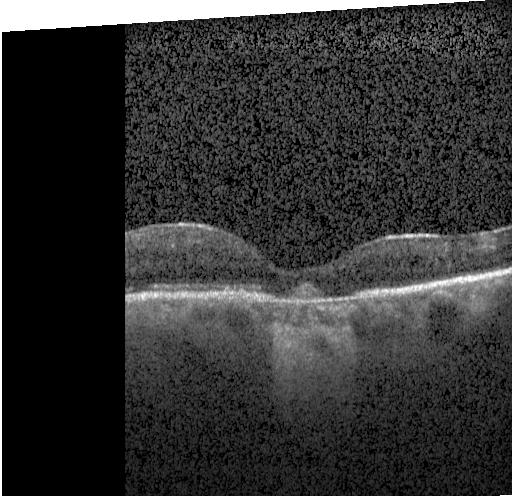 SD-OCT, OCT line scan. Finding: choroidal neovascularization.